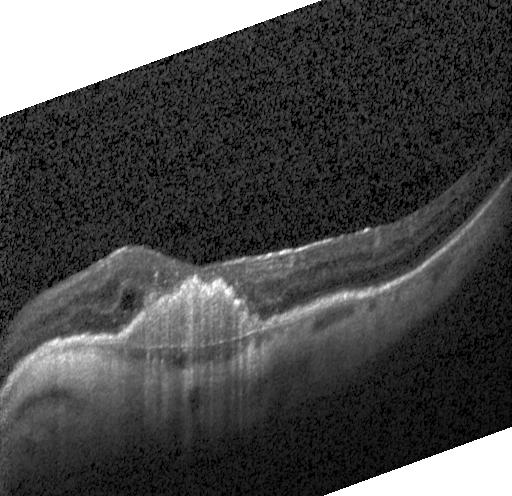 SD-OCT. Fovea-centered. OCT B-scan
Impression: choroidal neovascularization.